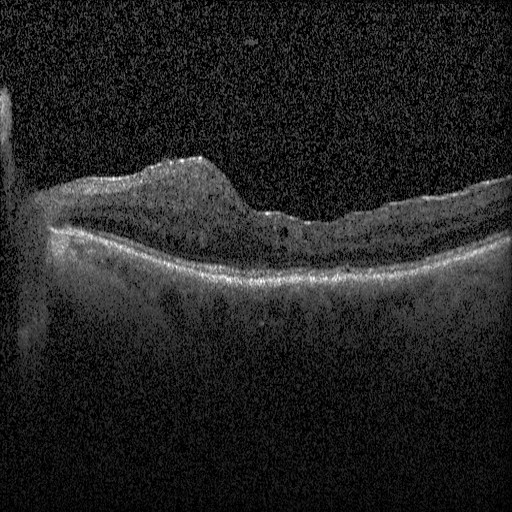

OCT finding: diabetic macular edema.